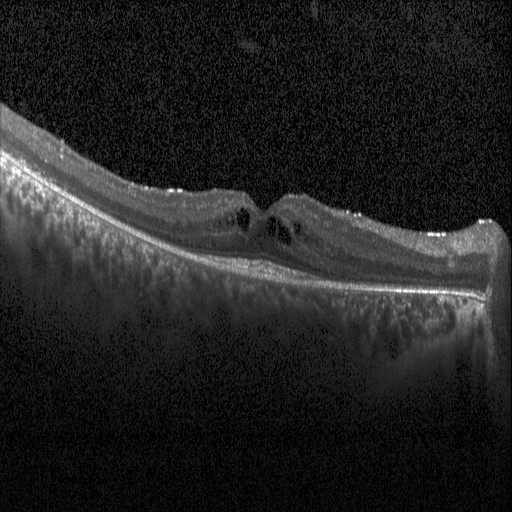 Horizontal scan through the fovea · SD-OCT · retinal OCT cross-section. Finding: diabetic macular edema (DME).